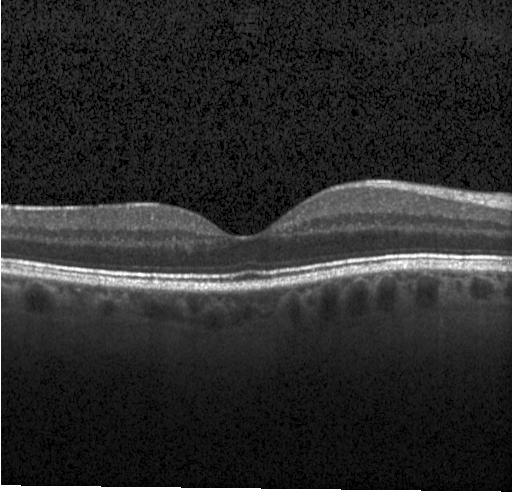

Impression: no choroidal neovascularization, no diabetic macular edema, and no drusen.